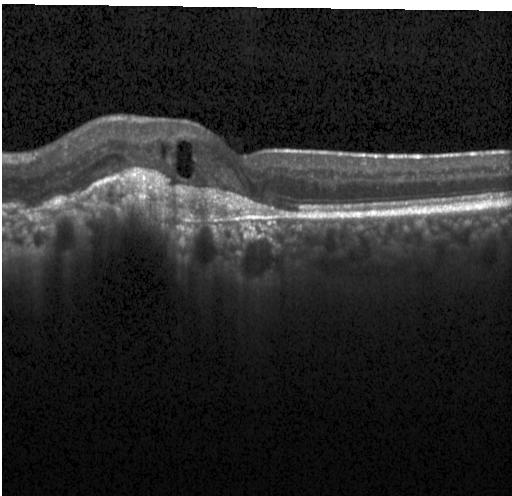

OCT finding: a choroidal neovascular membrane.